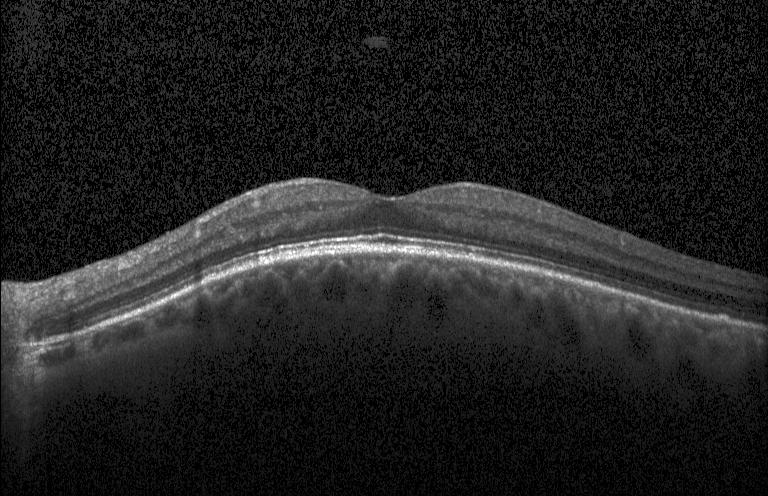
OCT line scan, horizontal scan through the fovea, spectral-domain optical coherence tomography. This B-scan demonstrates no CNV, DME, or drusen.